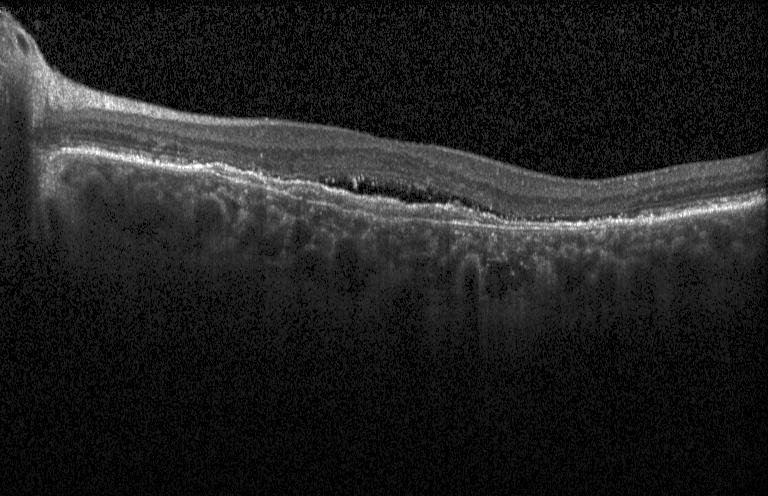

Centered on the fovea. SD-OCT. Retinal OCT cross-section — Diagnosis: choroidal neovascularization (CNV).